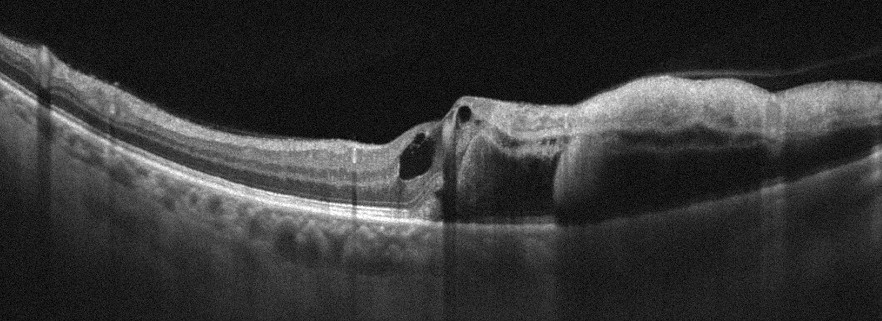 OCT line scan — Impression: retinal artery occlusion.